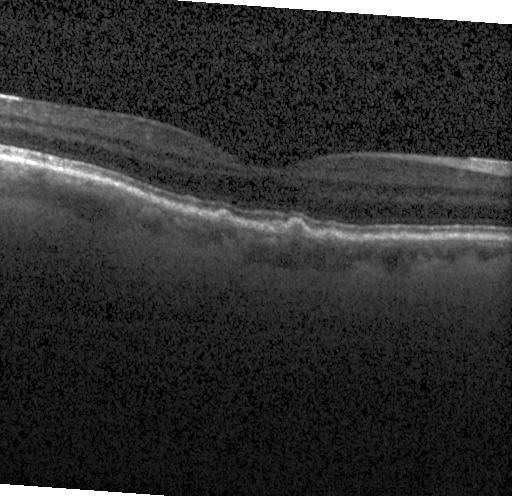 SD-OCT, retinal OCT B-scan, instrument: Heidelberg Spectralis, centered on the fovea.
The scan shows multiple drusen.